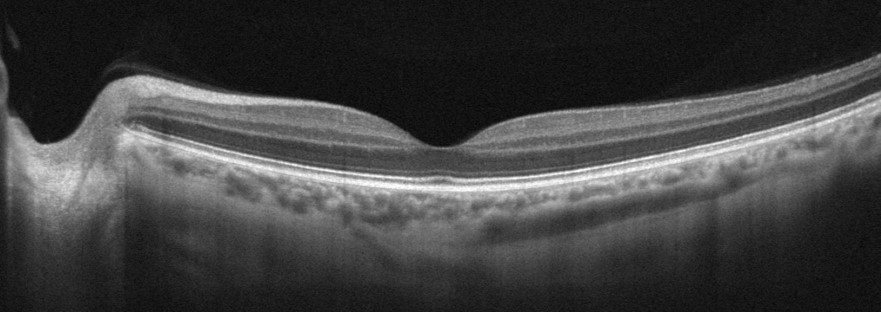 OCT B-scan showing no evidence of AMD, DME, ERM, RAO, RVO, or VID.